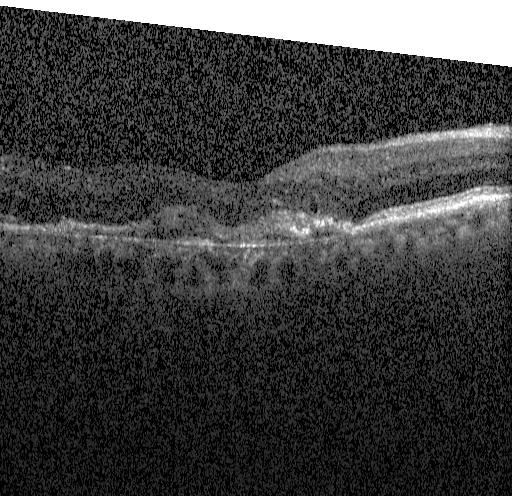 Dx: CNV.